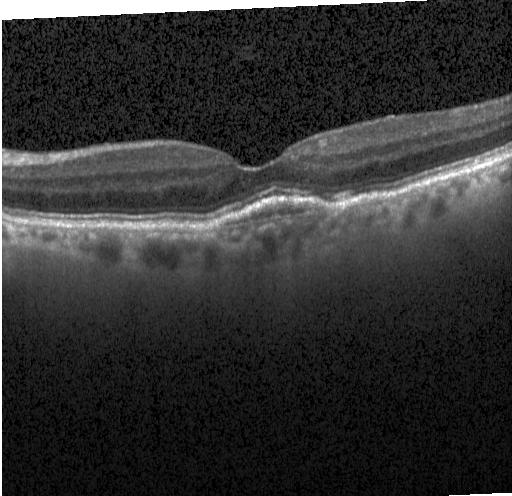
Diagnosis: a choroidal neovascular membrane.